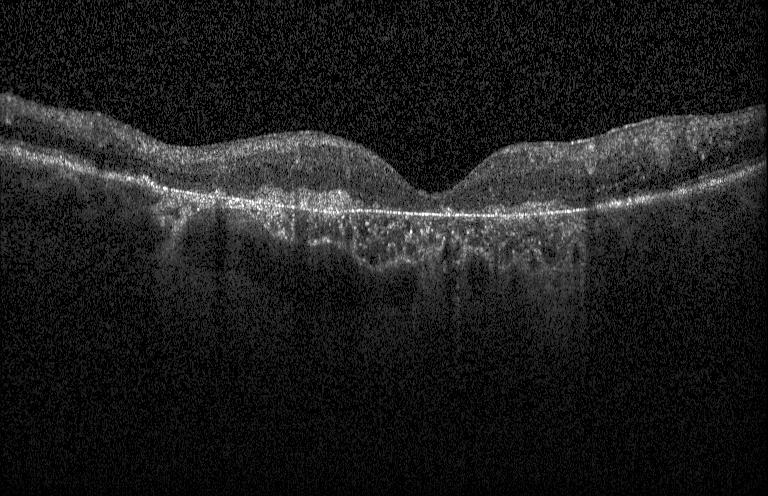
Optical coherence tomography scan. Finding: choroidal neovascularization.